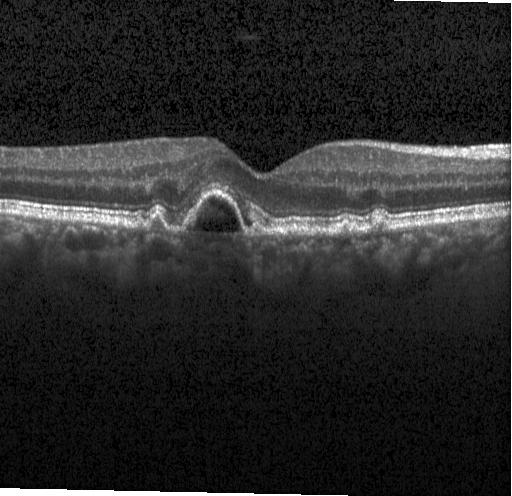

Spectral-domain optical coherence tomography · instrument: Heidelberg Spectralis · OCT line scan.
This B-scan demonstrates CNV.